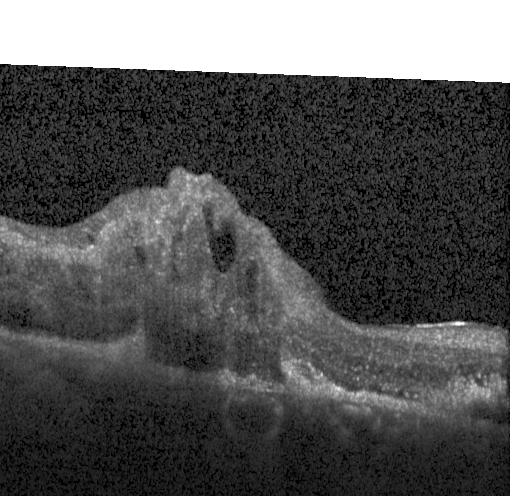 Horizontal scan through the fovea, OCT B-scan. Finding: CNV.